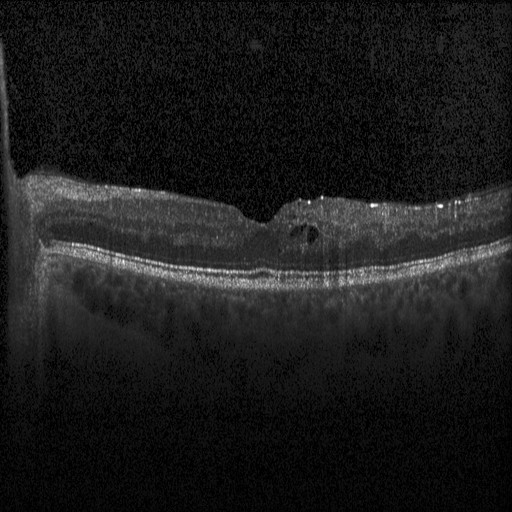 SD-OCT; OCT line scan; centered on the fovea — OCT finding: diabetic macular edema (DME).